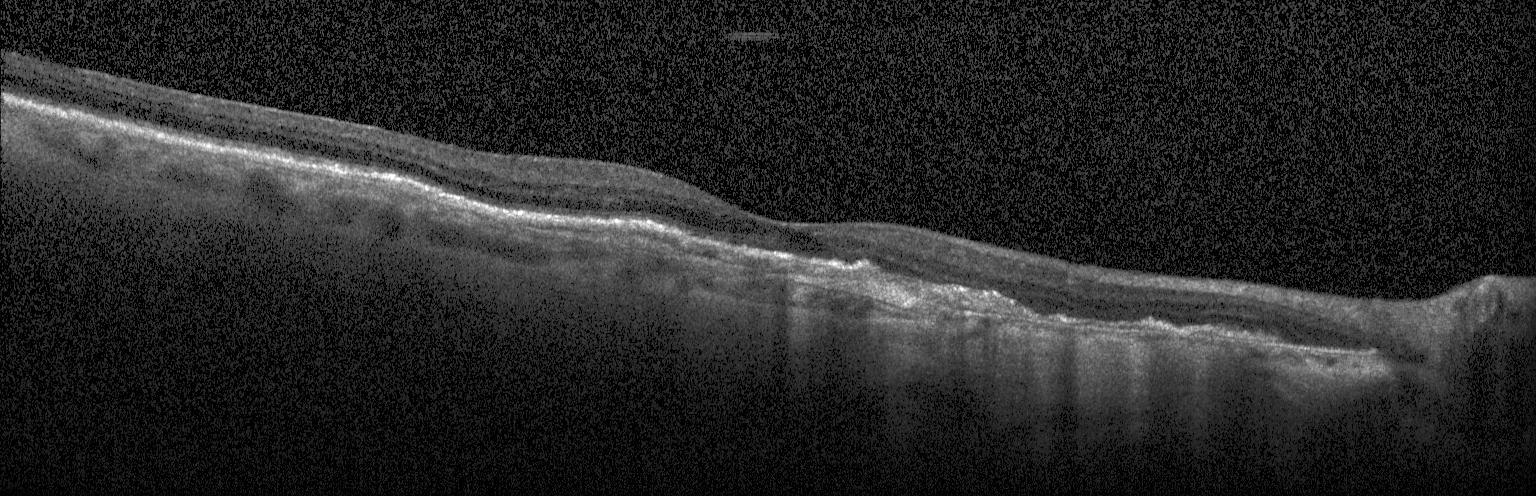

The scan shows a choroidal neovascular membrane.